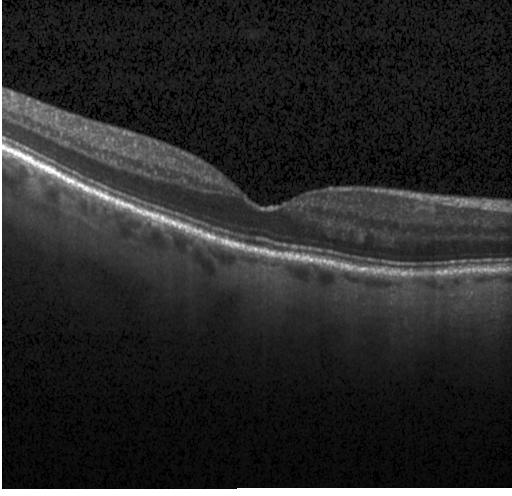
Optical coherence tomography B-scan, fovea-centered — Impression: no evidence of choroidal neovascularization, diabetic macular edema, or drusen.